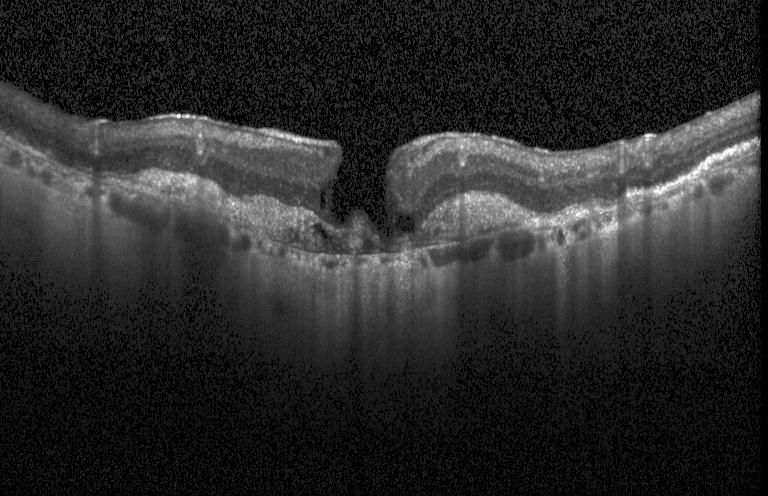

Choroidal neovascularization (CNV).